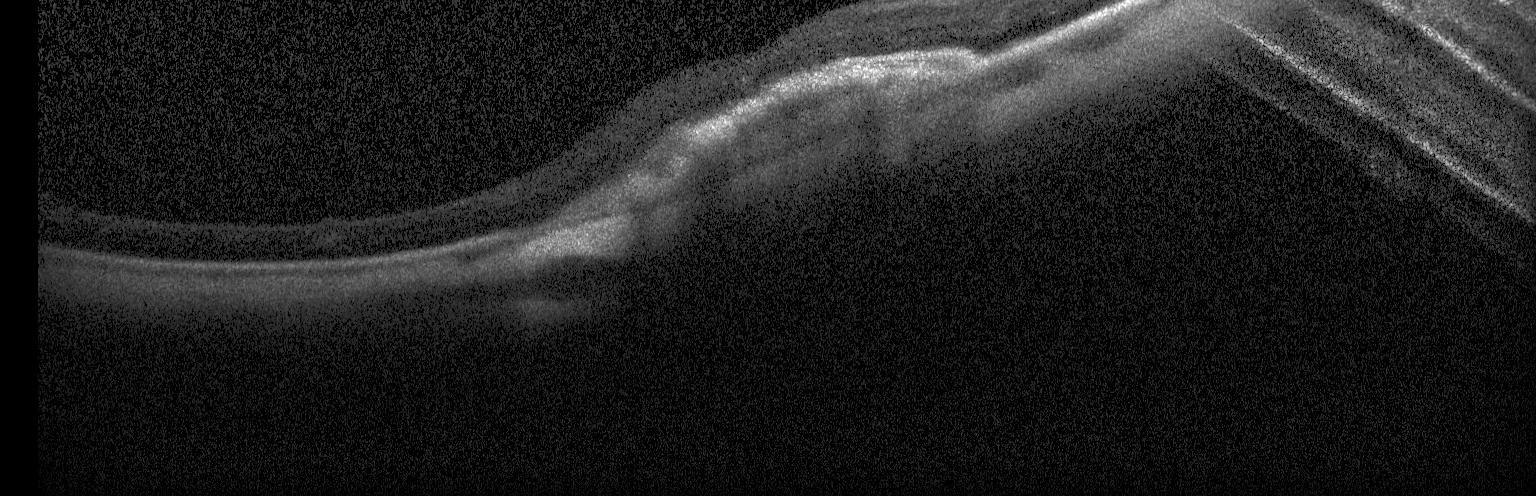 Optical coherence tomography scan · spectral-domain OCT · through the macula
Finding: a choroidal neovascular membrane.